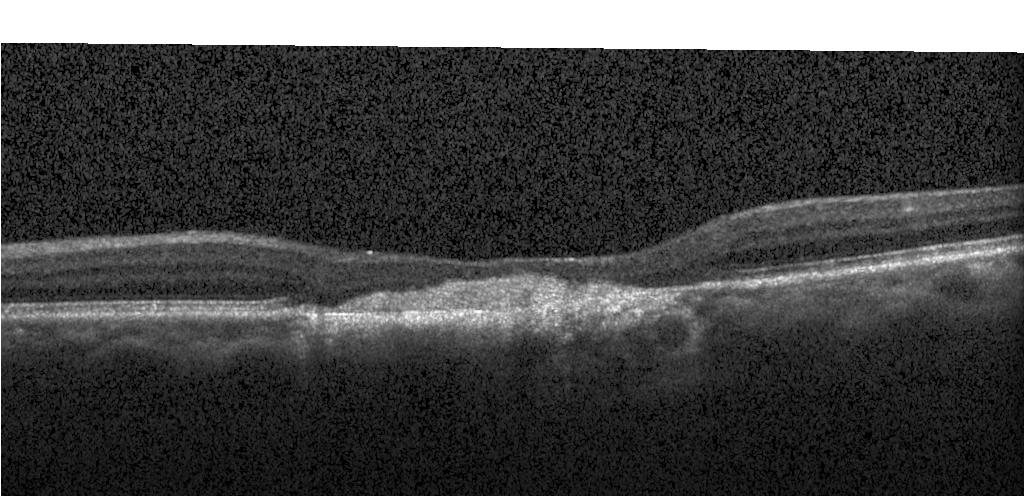

OCT B-scan.
Assessment: a choroidal neovascular membrane.